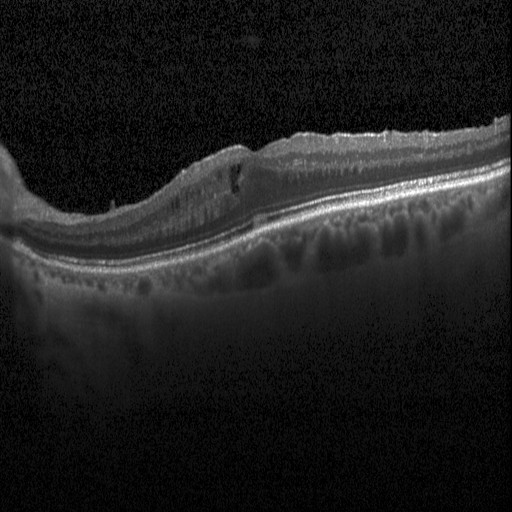

OCT B-scan. Diabetic macular edema.